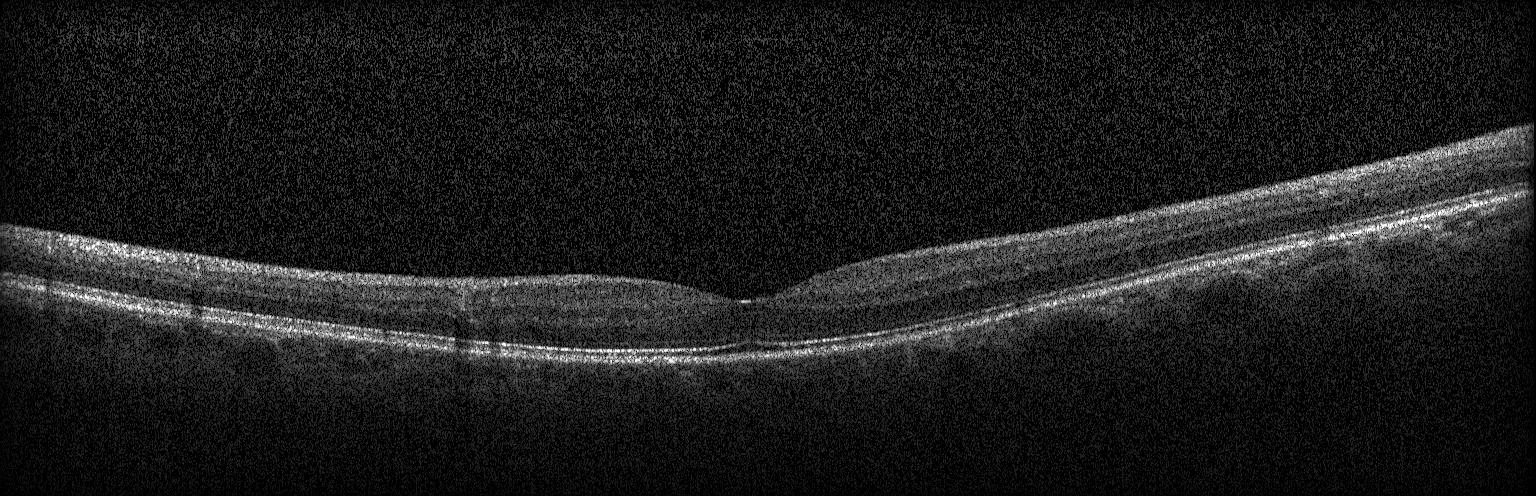
OCT B-scan — Diagnosis: no evidence of choroidal neovascularization, diabetic macular edema, or drusen.